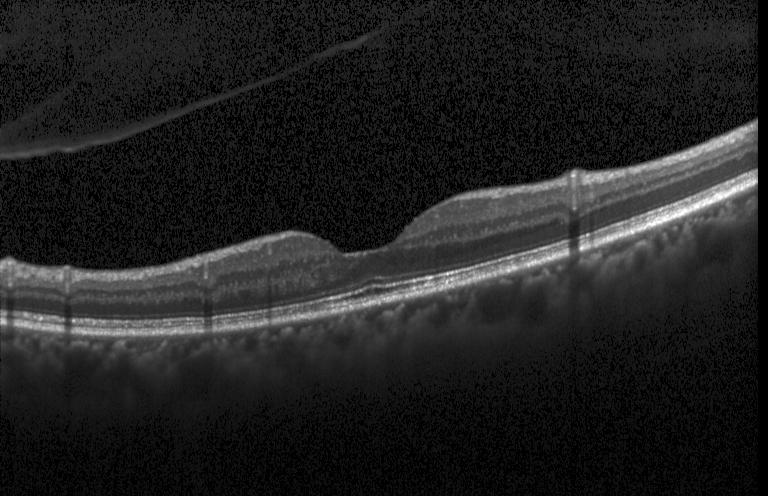 OCT B-scan showing neither choroidal neovascularization, diabetic macular edema, nor drusen.